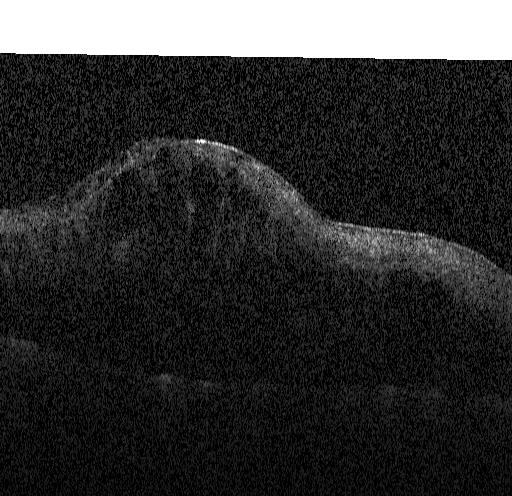 Macular OCT: DME.